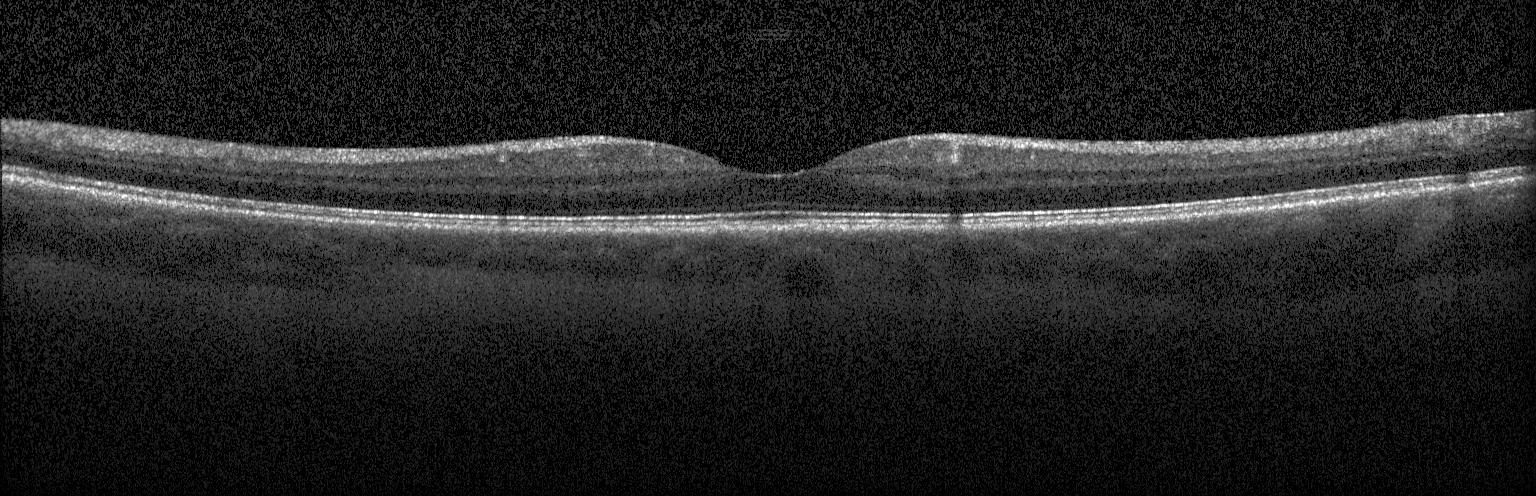
Heidelberg Spectralis OCT system · optical coherence tomography B-scan · spectral-domain optical coherence tomography.
No evidence of choroidal neovascularization, diabetic macular edema, or drusen.